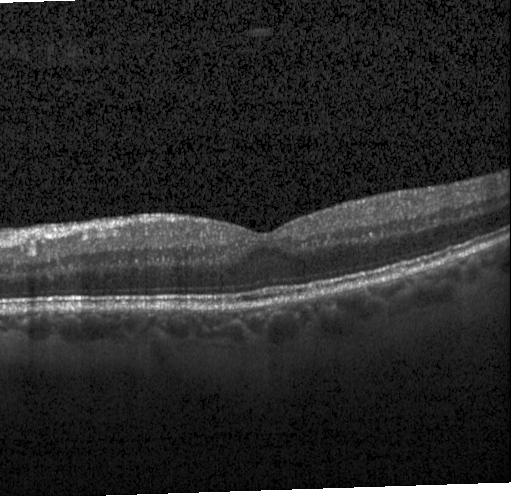
This B-scan demonstrates no choroidal neovascularization, no diabetic macular edema, and no drusen.